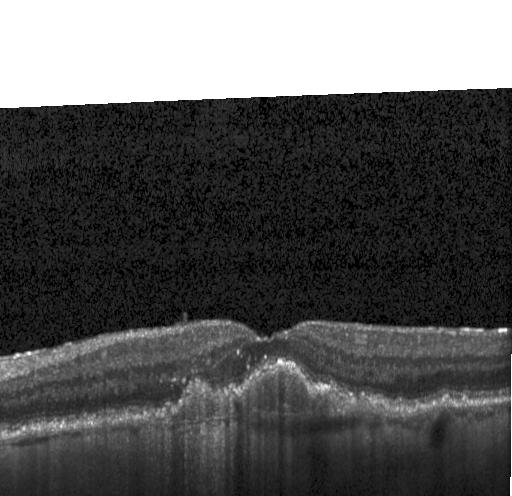

Heidelberg Spectralis; SD-OCT; OCT B-scan
Impression: choroidal neovascularization.